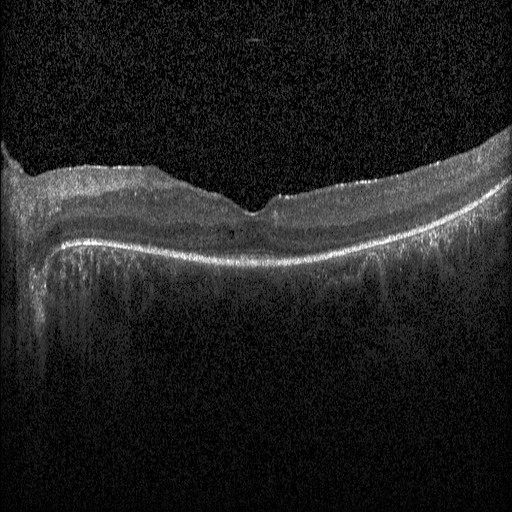
Assessment: diabetic macular edema.